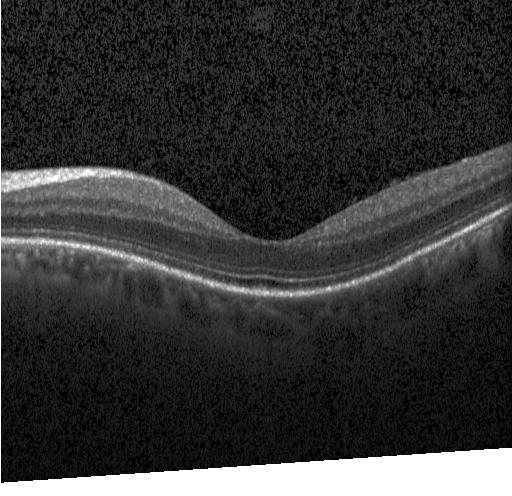 Impression: neither CNV, DME, nor drusen.